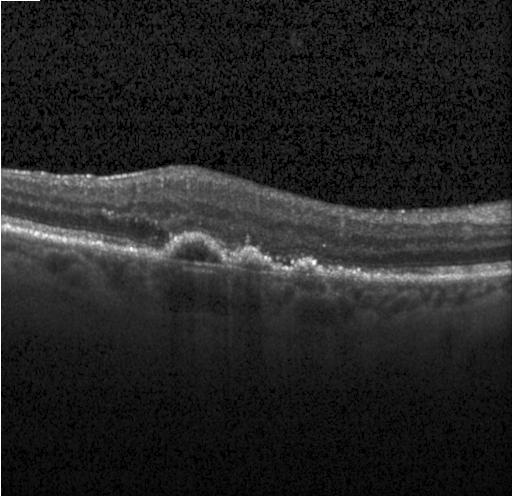 OCT finding: a choroidal neovascular membrane.